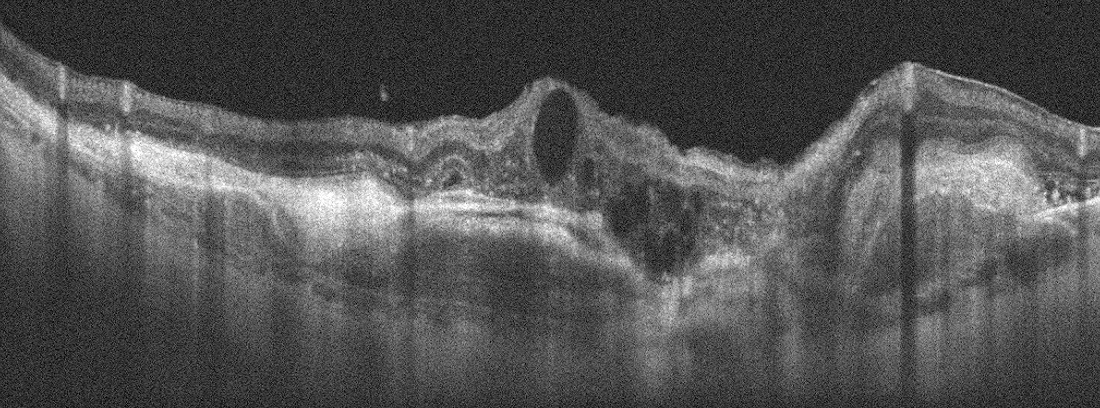 OCT B-scan — Diagnosis: age-related macular degeneration.